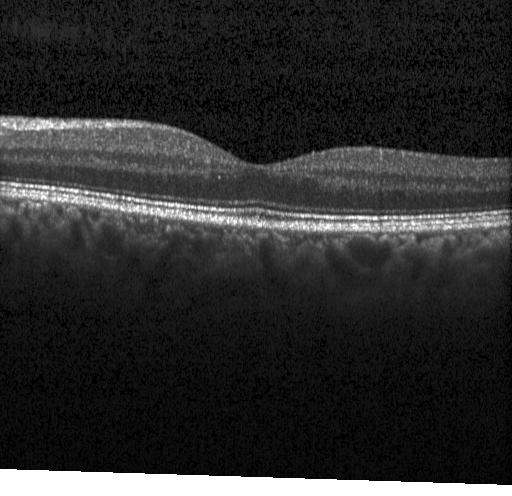 Diagnosis: no choroidal neovascularization, diabetic macular edema, or drusen.